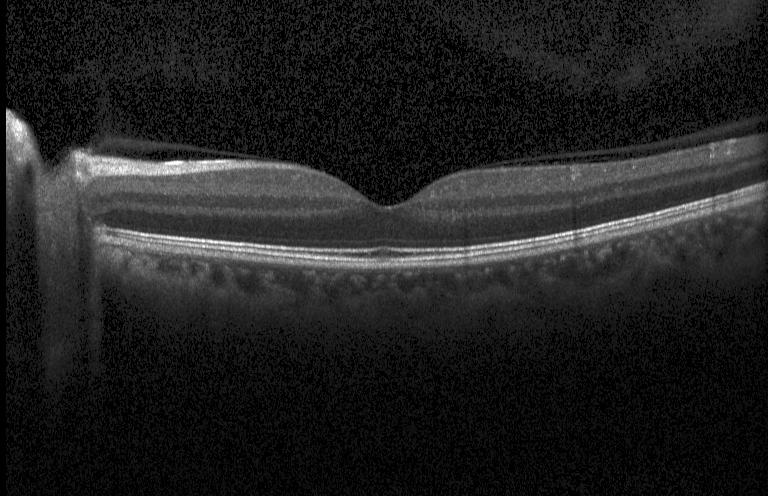
OCT line scan — Finding: no CNV, no DME, and no drusen.